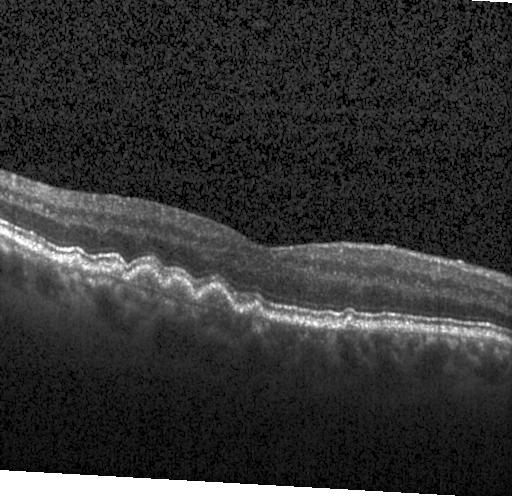 Macular scan · optical coherence tomography scan · acquired on a Heidelberg Spectralis · SD-OCT — Impression: drusen.